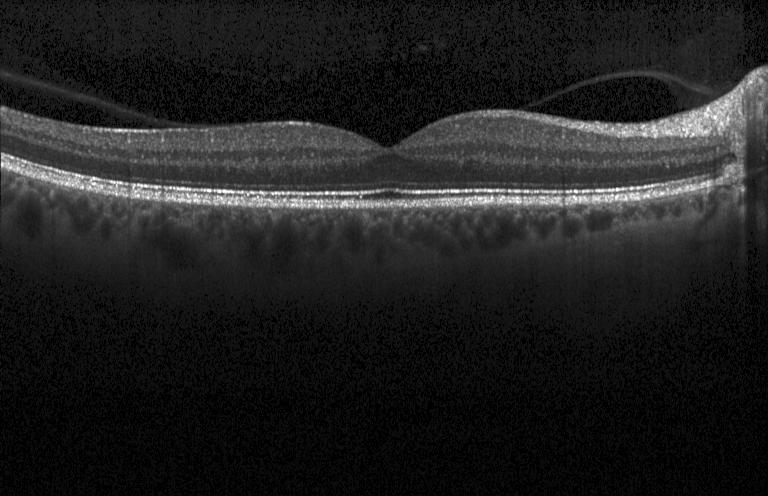

Optical coherence tomography B-scan, spectral-domain optical coherence tomography. Assessment: no CNV, no DME, and no drusen.